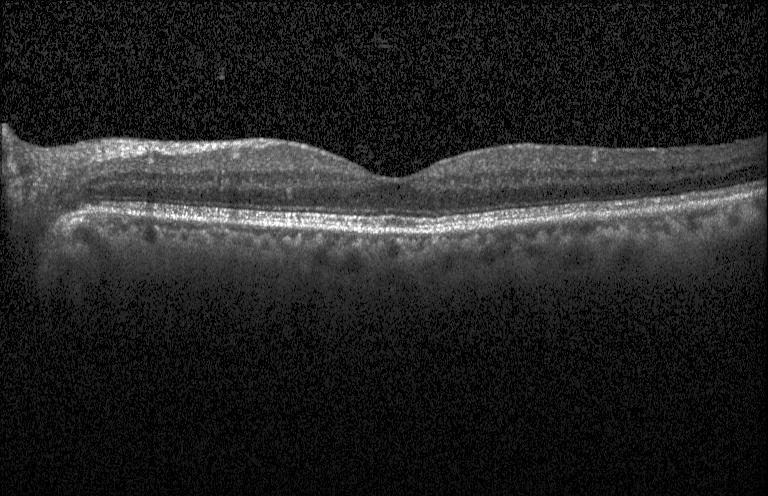

Diagnosis: no evidence of choroidal neovascularization, diabetic macular edema, or drusen.